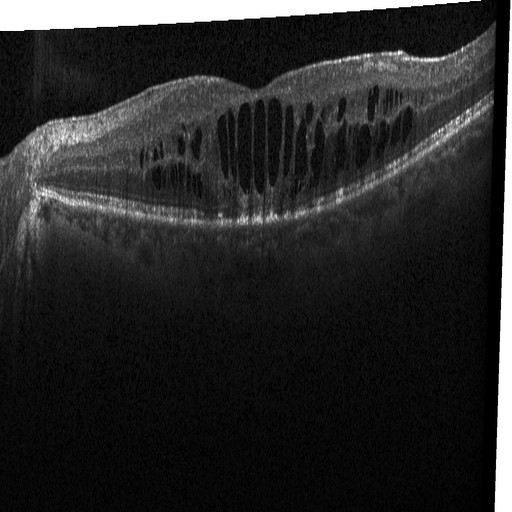
Retinal OCT B-scan · horizontal scan through the fovea · SD-OCT. DME.